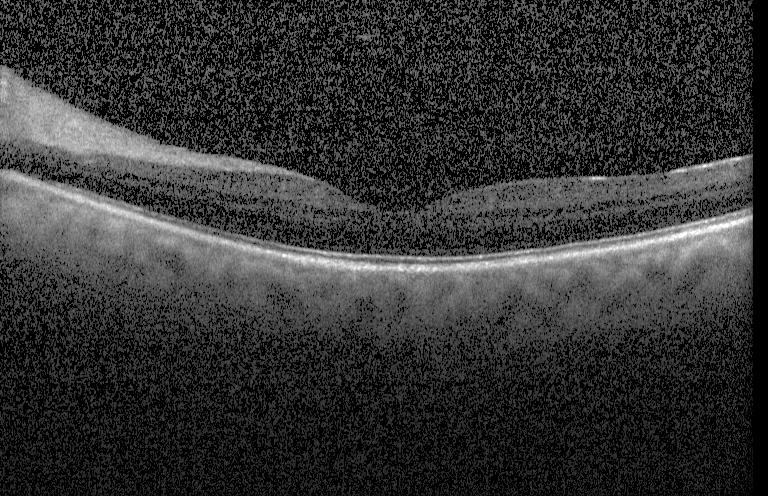 OCT B-scan.
No evidence of CNV, DME, or drusen.